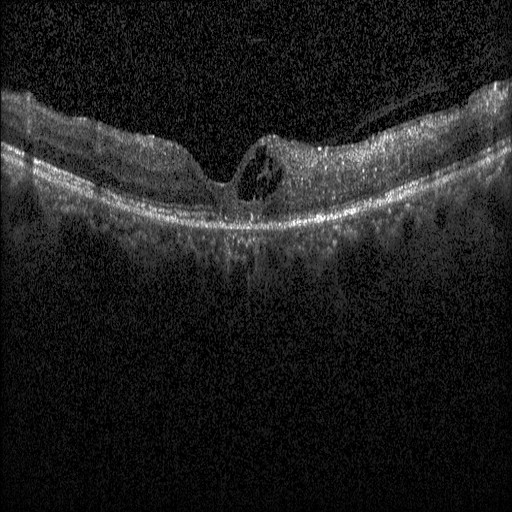 Macular OCT: DME.